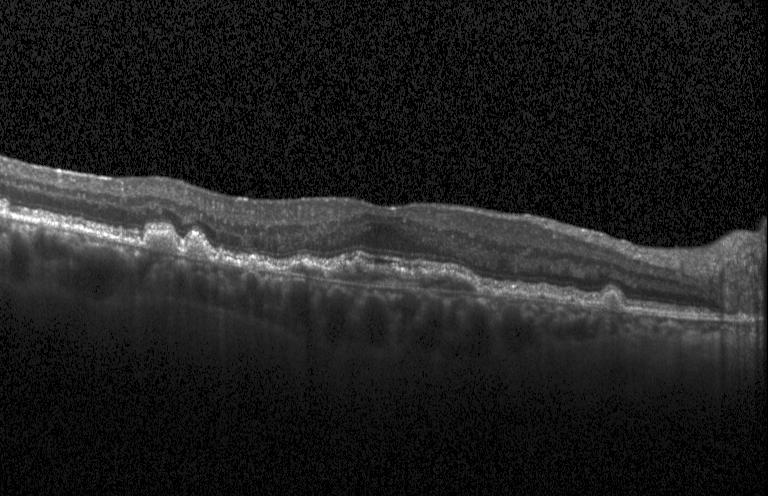
OCT B-scan; spectral-domain OCT — CNV.